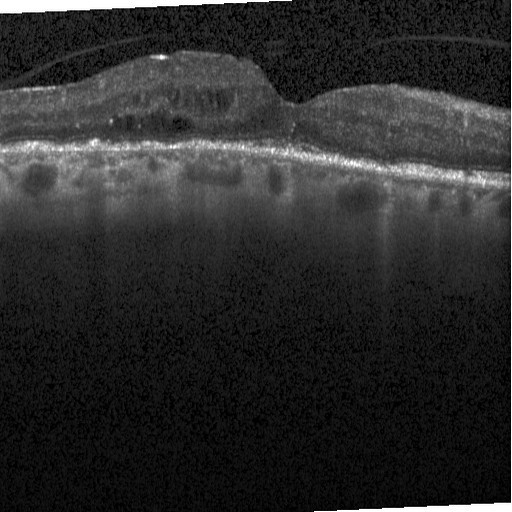

This B-scan demonstrates diabetic macular edema (DME).